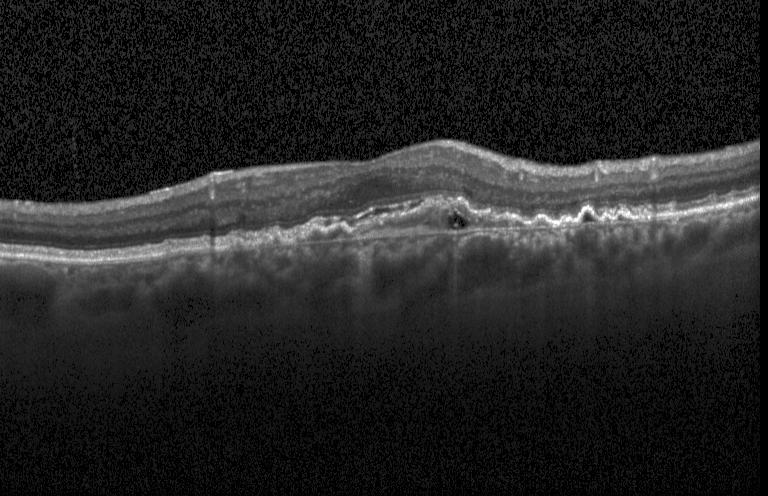
Spectral-domain OCT, retinal OCT cross-section, fovea-centered, Heidelberg Spectralis
This B-scan demonstrates a choroidal neovascular membrane.